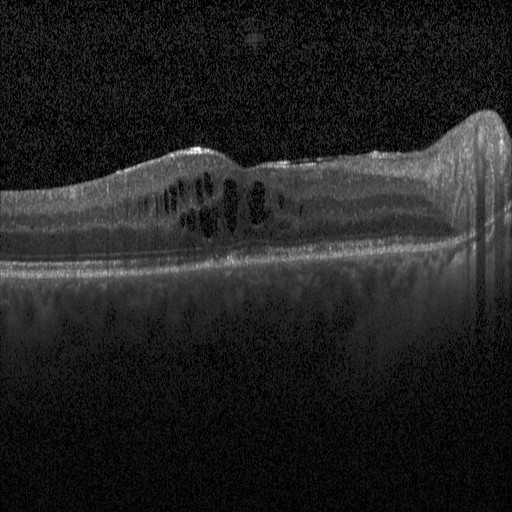
Spectral-domain optical coherence tomography, centered on the fovea, Heidelberg Spectralis, OCT line scan — OCT finding: diabetic macular edema (DME).